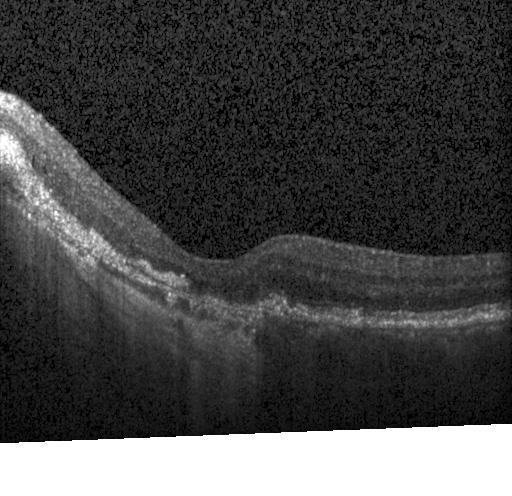

The scan shows a choroidal neovascular membrane.